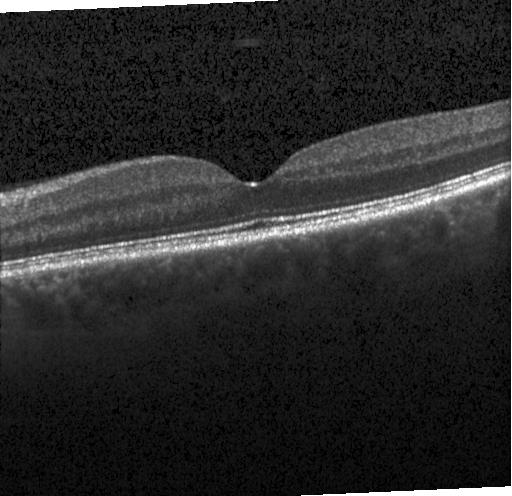

OCT scan showing neither choroidal neovascularization, diabetic macular edema, nor drusen.